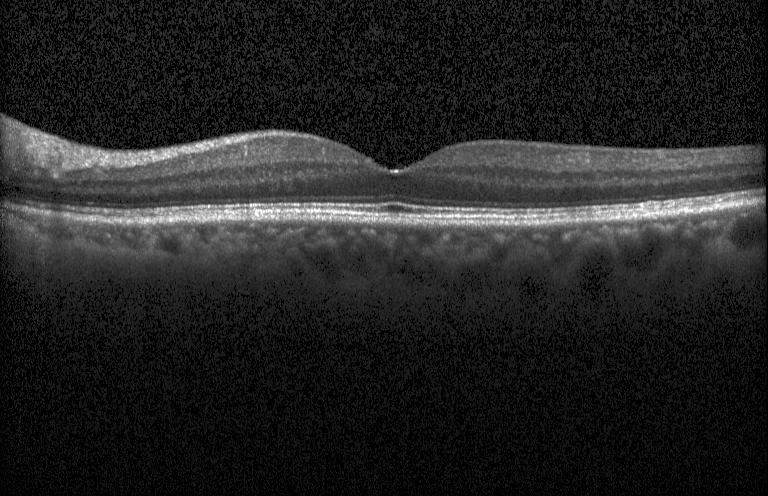

Retinal OCT B-scan · SD-OCT · macular scan · Heidelberg Spectralis. This B-scan demonstrates no evidence of CNV, DME, or drusen.